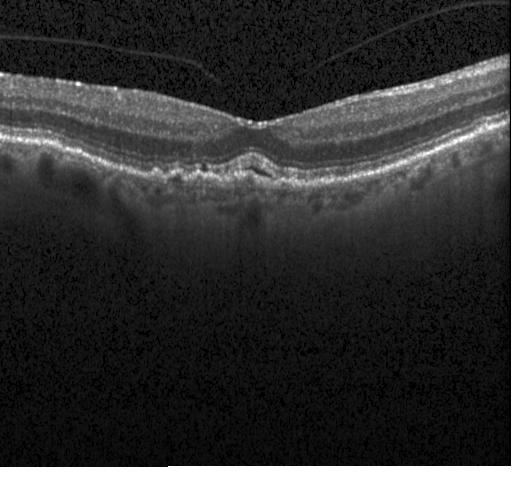

OCT B-scan · SD-OCT. Assessment: a choroidal neovascular membrane.